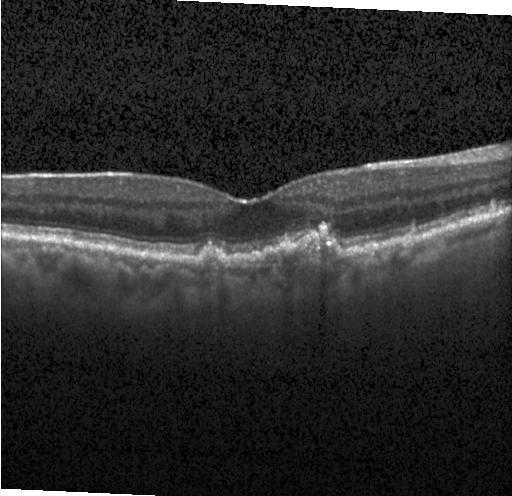
Retinal OCT cross-section — The scan shows a choroidal neovascular membrane.